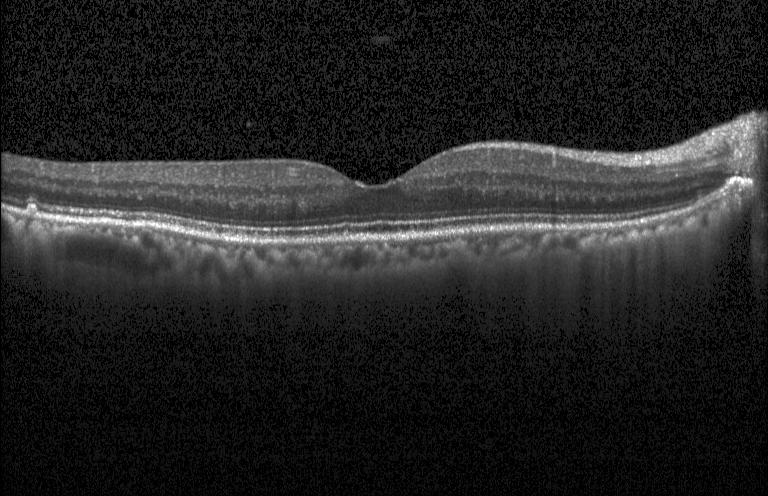
Fovea-centered. Retinal OCT B-scan. Instrument: Heidelberg Spectralis — The scan shows no CNV, no DME, and no drusen.